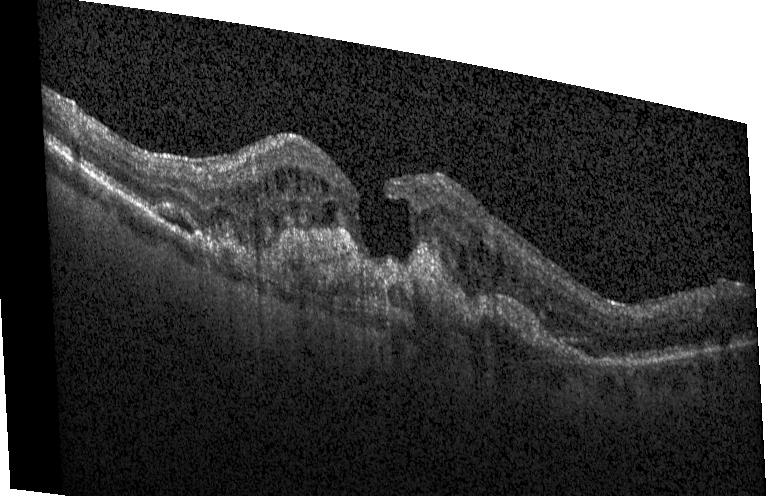 Macular scan. Optical coherence tomography B-scan. Instrument: Heidelberg Spectralis. Spectral-domain optical coherence tomography
Diagnosis: choroidal neovascularization.